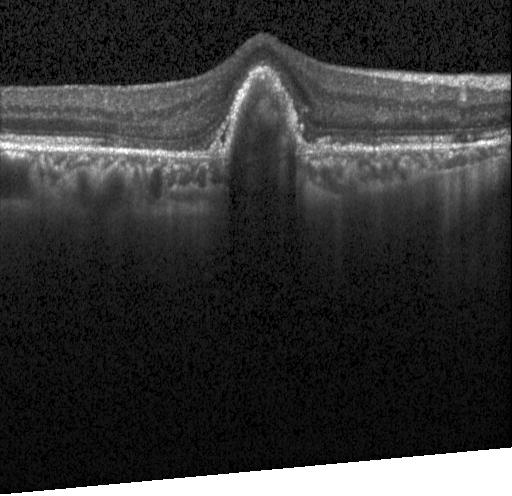
Finding: a choroidal neovascular membrane.